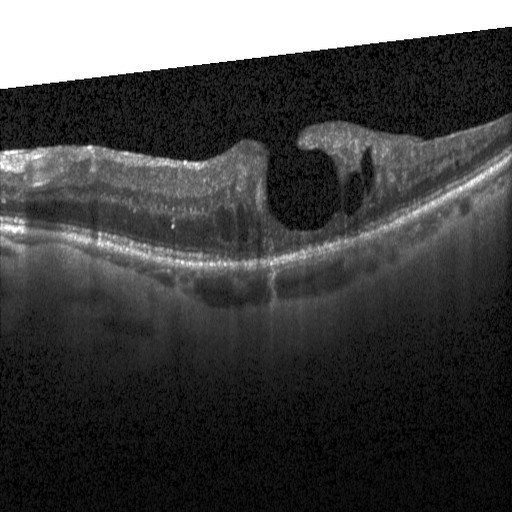
Spectral-domain OCT; OCT line scan. Macular OCT: diabetic macular edema (DME).